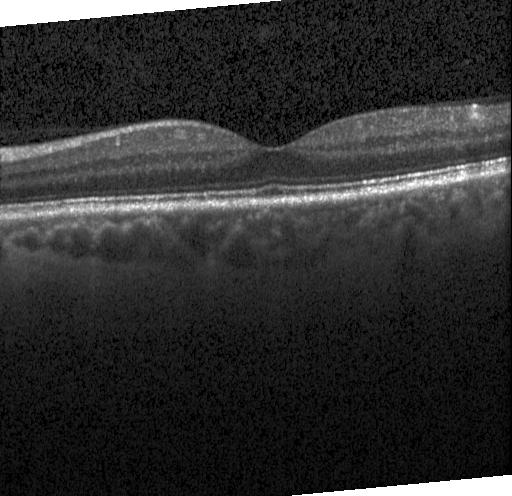
Dx: neither choroidal neovascularization, diabetic macular edema, nor drusen.